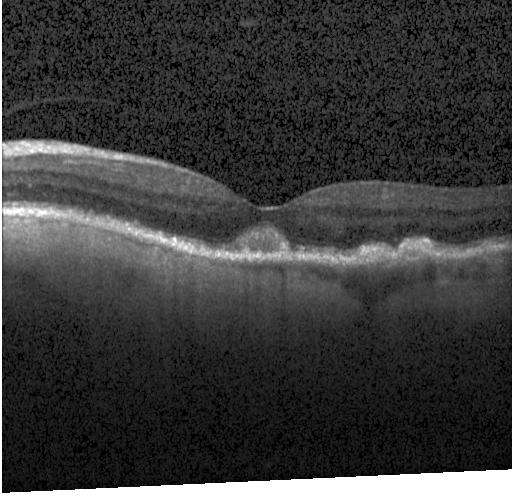

Centered on the fovea; OCT B-scan — Dx: sub-RPE drusenoid deposits.